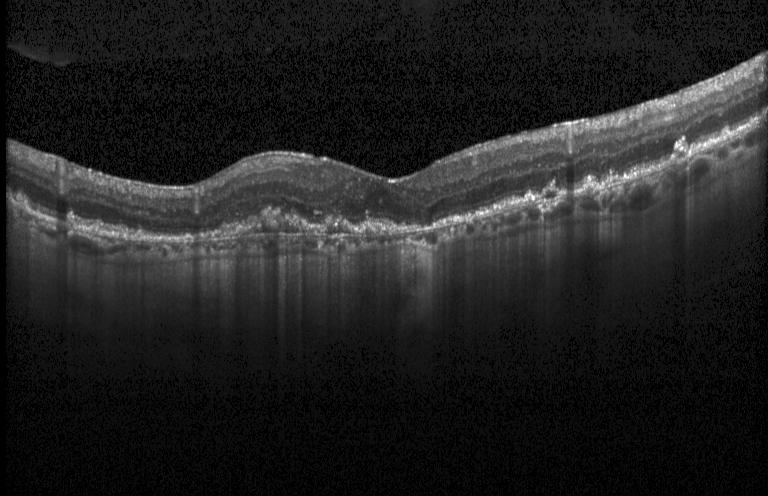
Retinal OCT B-scan — Assessment: a choroidal neovascular membrane.